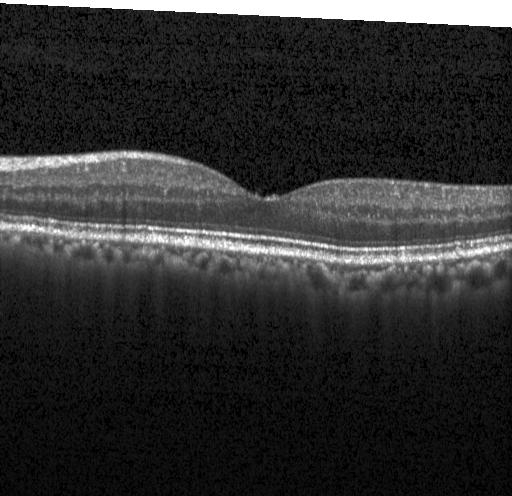

OCT finding: no evidence of CNV, DME, or drusen.